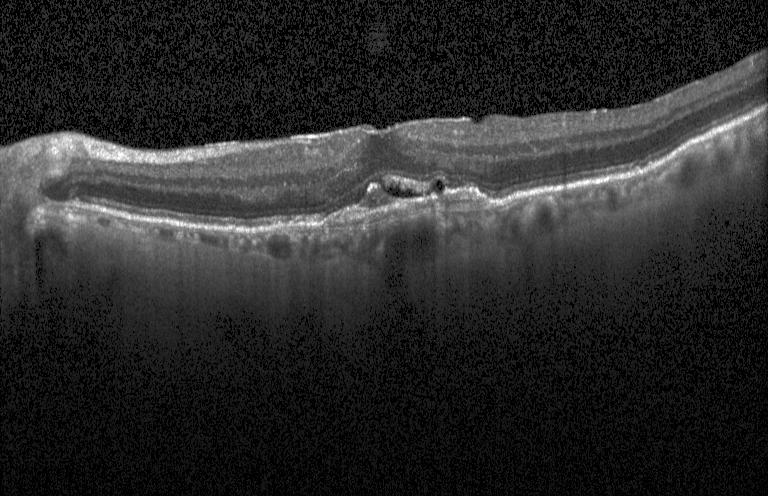

Retinal OCT B-scan; SD-OCT; Heidelberg Spectralis
Finding: choroidal neovascularization (CNV).